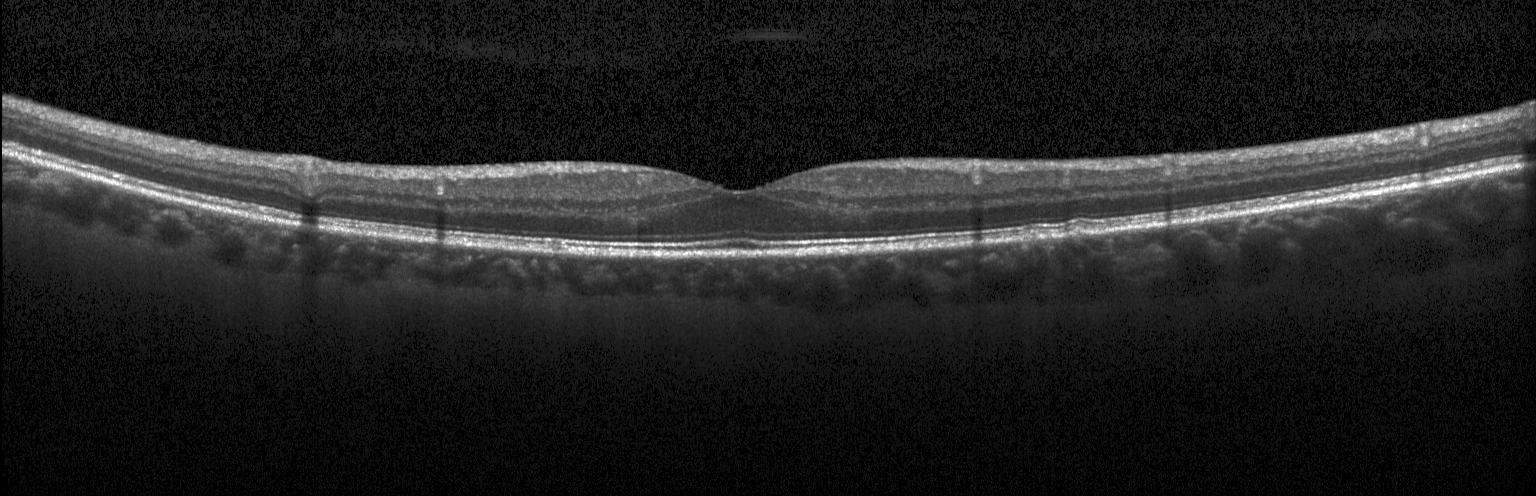
Through the macula · retinal OCT B-scan · instrument: Heidelberg Spectralis.
Impression: no evidence of choroidal neovascularization, diabetic macular edema, or drusen.